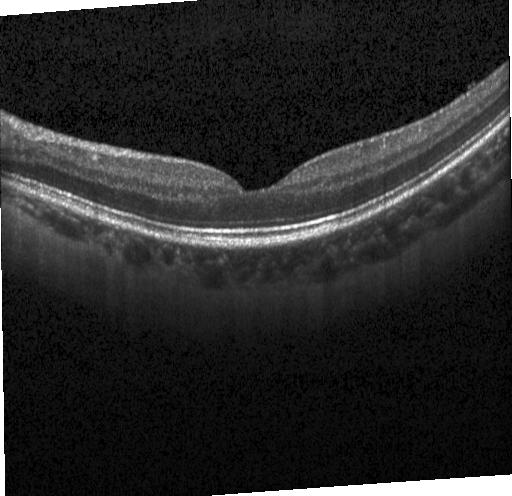
Optical coherence tomography B-scan, spectral-domain optical coherence tomography, Heidelberg Spectralis OCT system, macular scan. Diagnosis: neither choroidal neovascularization, diabetic macular edema, nor drusen.